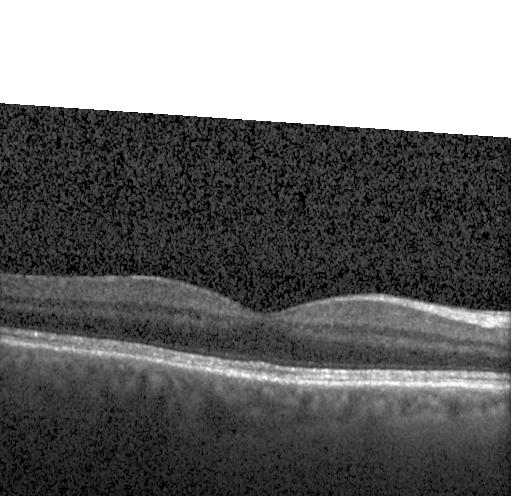

Retinal OCT cross-section; Heidelberg Spectralis OCT system; spectral-domain optical coherence tomography.
Finding: no CNV, DME, or drusen.